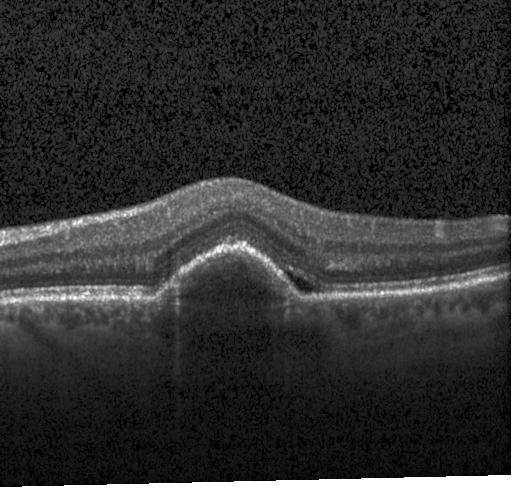

OCT B-scan.
Diagnosis: a choroidal neovascular membrane.